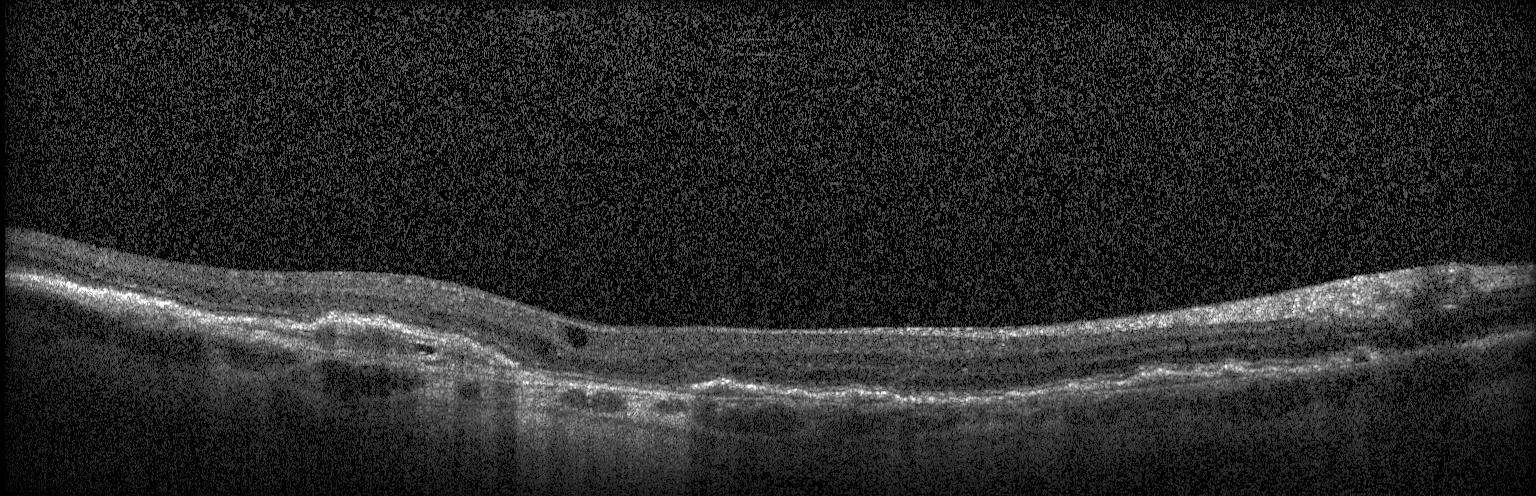 OCT scan showing a choroidal neovascular membrane.